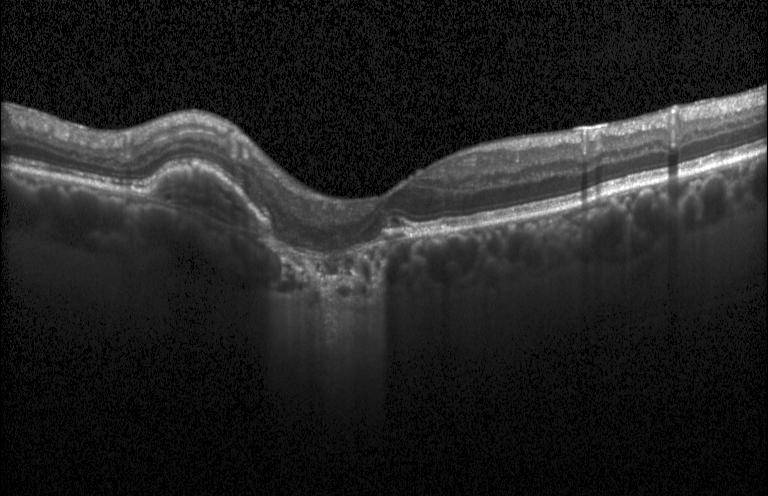

OCT B-scan, SD-OCT, fovea-centered, Heidelberg Spectralis
This B-scan demonstrates a choroidal neovascular membrane.